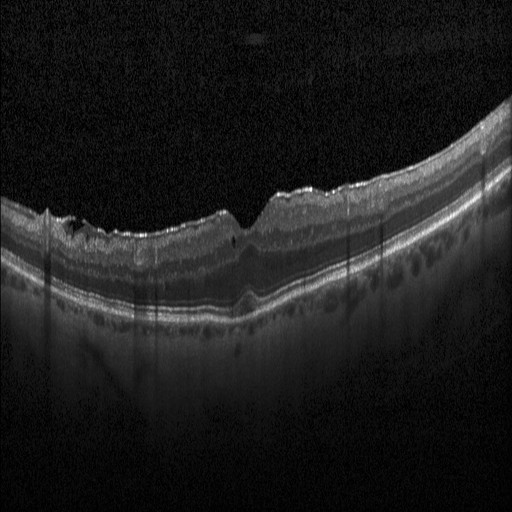
Impression: diabetic macular edema (DME).